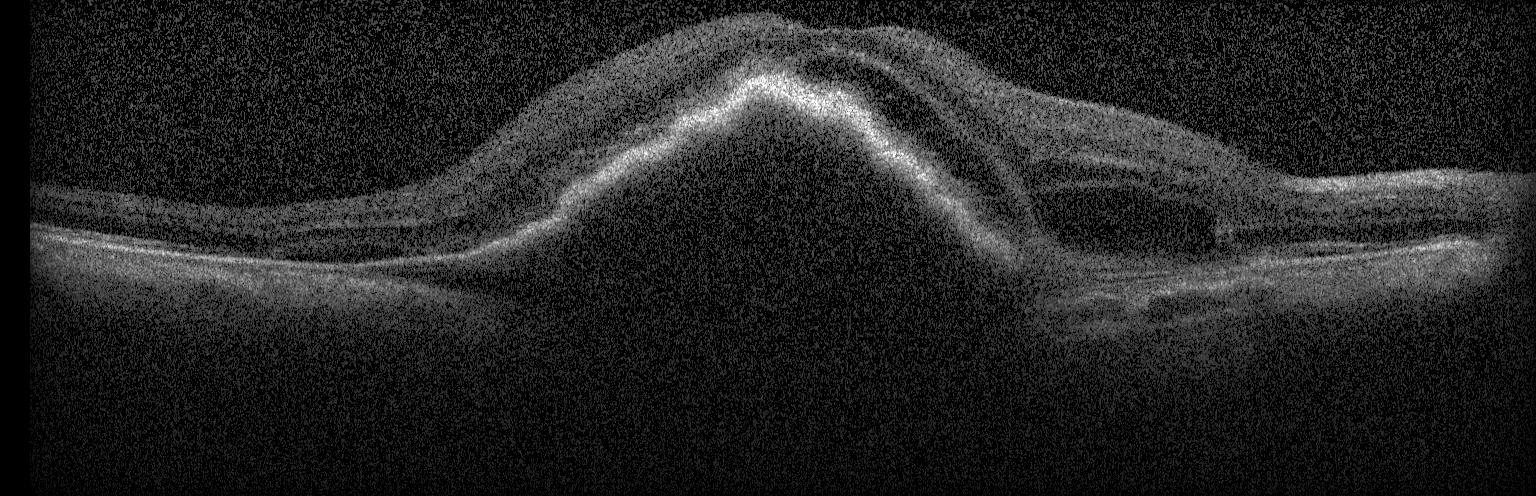

OCT line scan, Heidelberg Spectralis OCT system
This B-scan demonstrates a choroidal neovascular membrane.